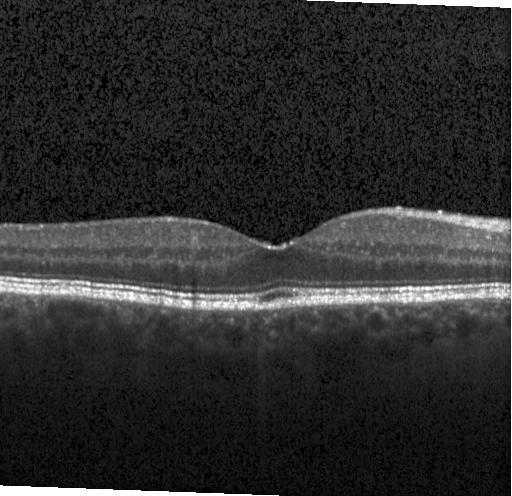

OCT B-scan. Spectral-domain OCT — Macular OCT: no CNV, DME, or drusen.